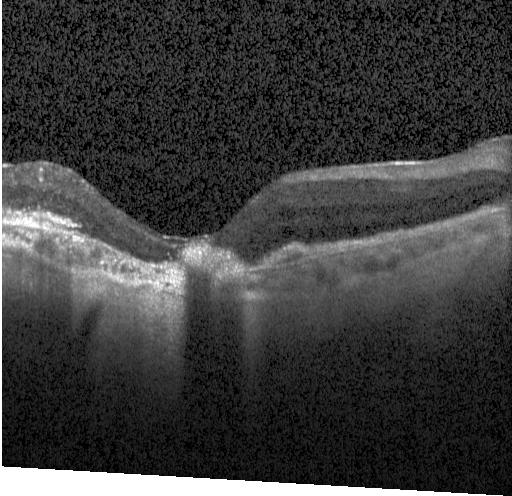 Diagnosis: a choroidal neovascular membrane.